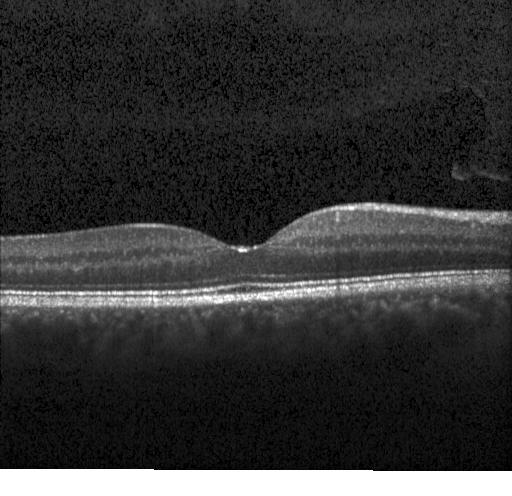 Macular OCT: neither choroidal neovascularization, diabetic macular edema, nor drusen.